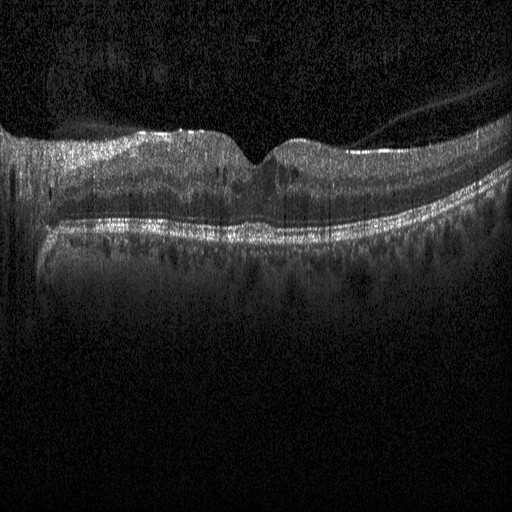
Retinal OCT cross-section; fovea-centered. Impression: diabetic macular edema (DME).